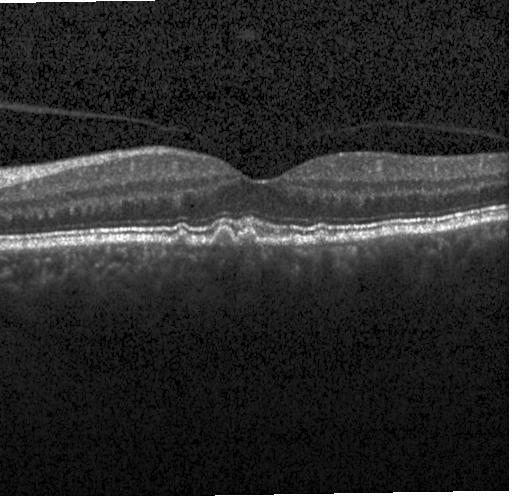 Optical coherence tomography scan · spectral-domain OCT · through the macula · Heidelberg Spectralis OCT system
Dx: sub-RPE drusenoid deposits.